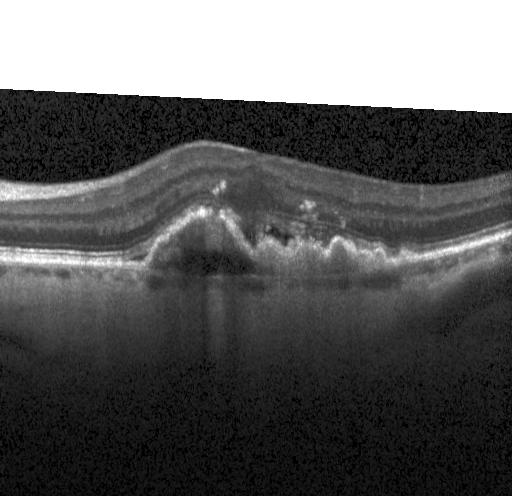
OCT B-scan. Diagnosis: a choroidal neovascular membrane.